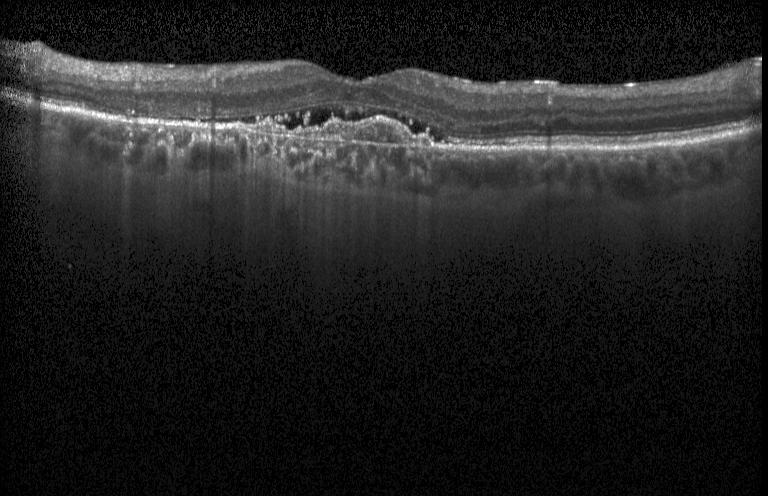
The scan shows a choroidal neovascular membrane.